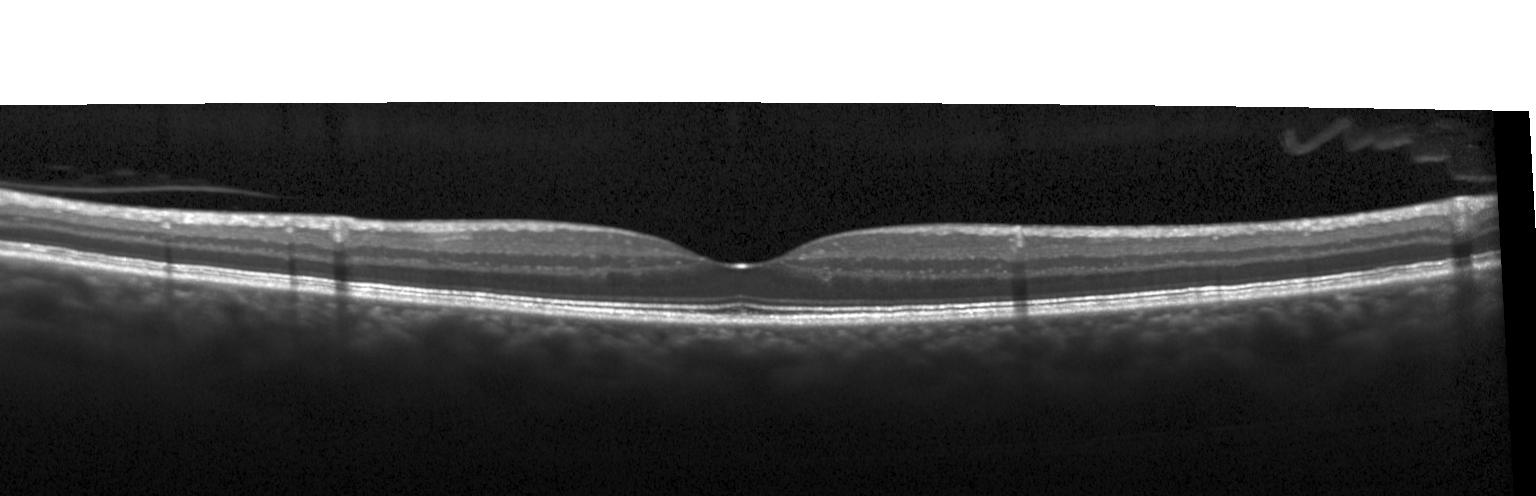

Retinal OCT B-scan. Macular scan. OCT finding: no choroidal neovascularization, no diabetic macular edema, and no drusen.